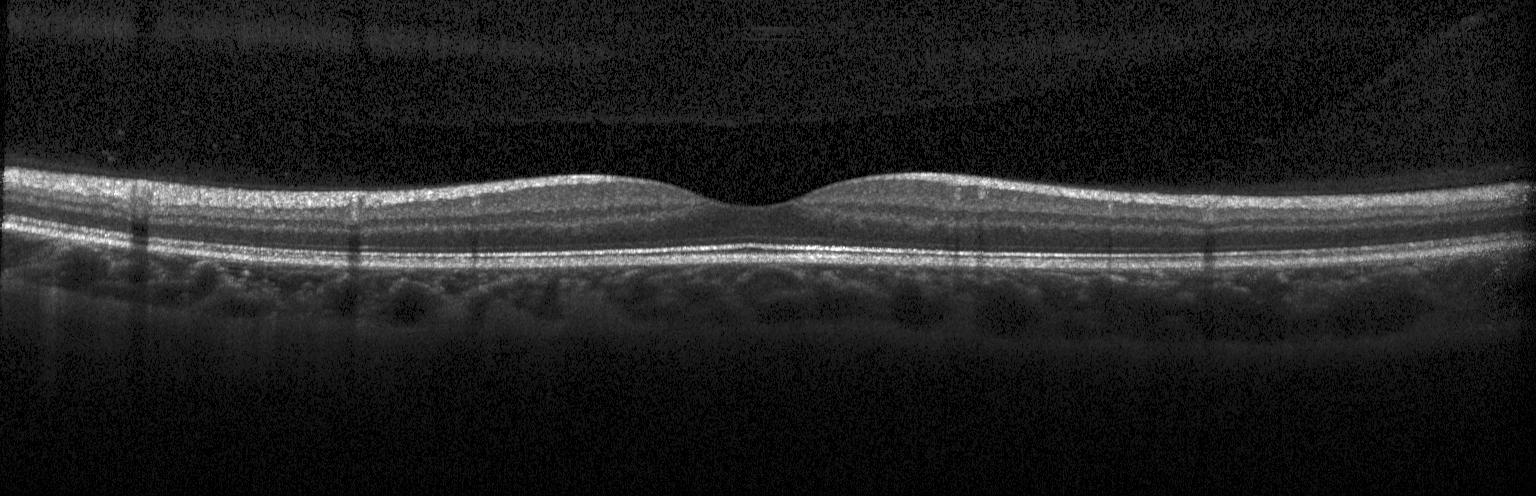
Retinal OCT cross-section — Diagnosis: neither choroidal neovascularization, diabetic macular edema, nor drusen.